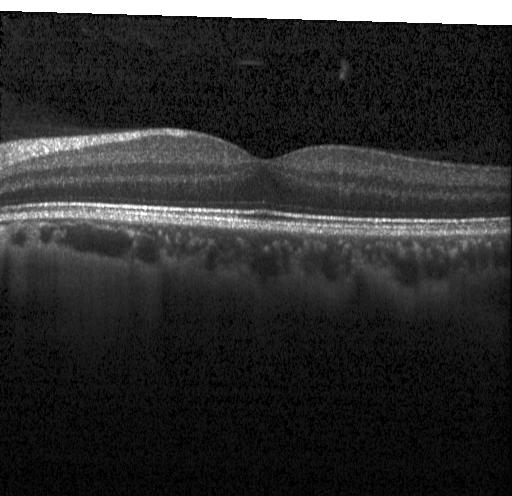 OCT B-scan, Heidelberg Spectralis.
Assessment: no choroidal neovascularization, diabetic macular edema, or drusen.